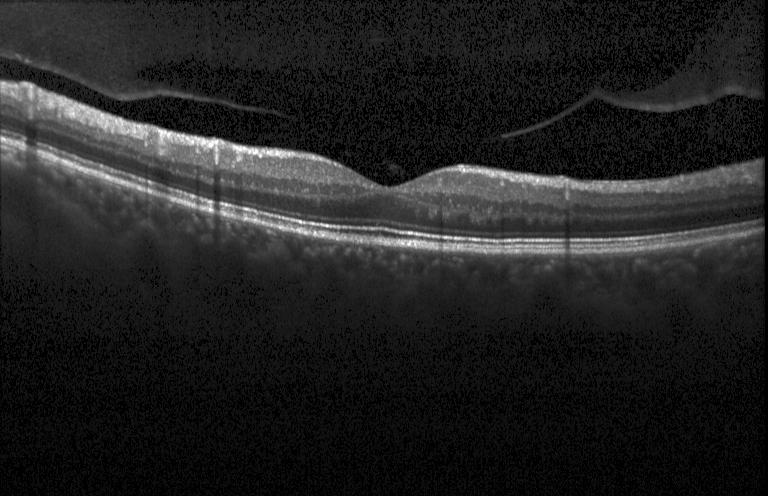

OCT B-scan. SD-OCT — Macular OCT: no choroidal neovascularization, no diabetic macular edema, and no drusen.